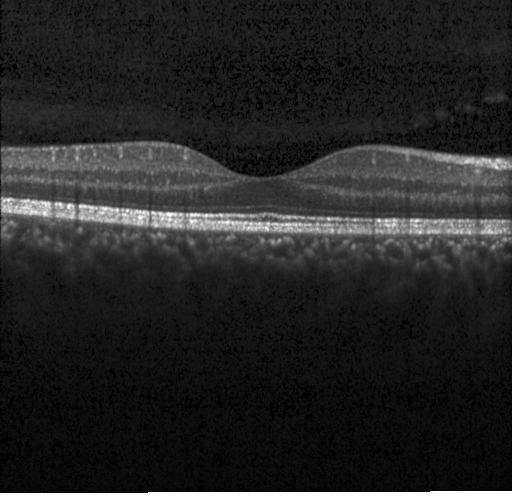 Spectral-domain optical coherence tomography · horizontal scan through the fovea · optical coherence tomography scan · instrument: Heidelberg Spectralis
Macular OCT: no evidence of CNV, DME, or drusen.